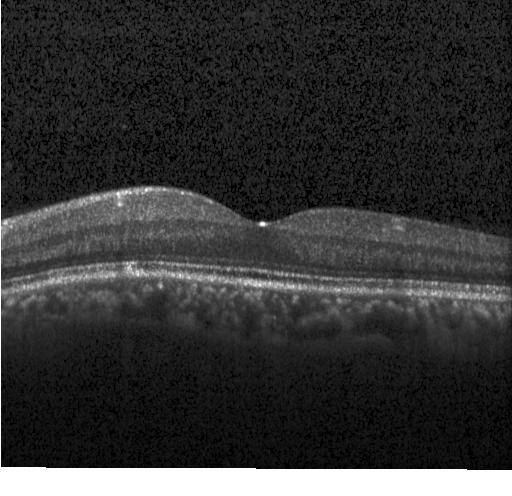 Finding: no choroidal neovascularization, no diabetic macular edema, and no drusen.